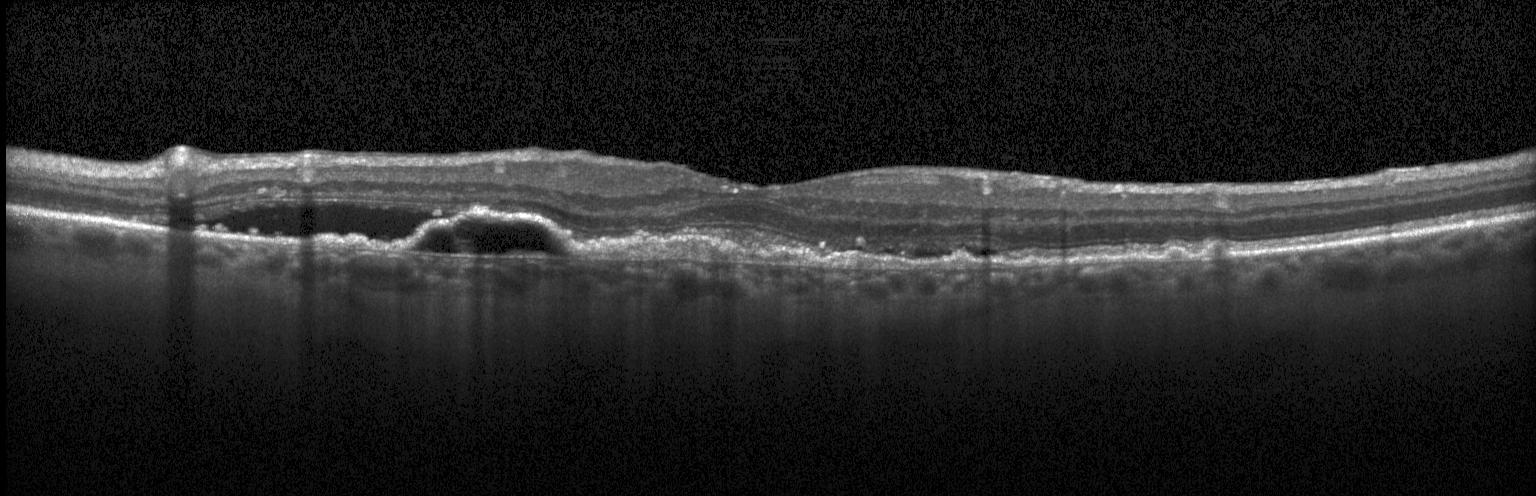 Retinal OCT cross-section.
The scan shows a choroidal neovascular membrane.